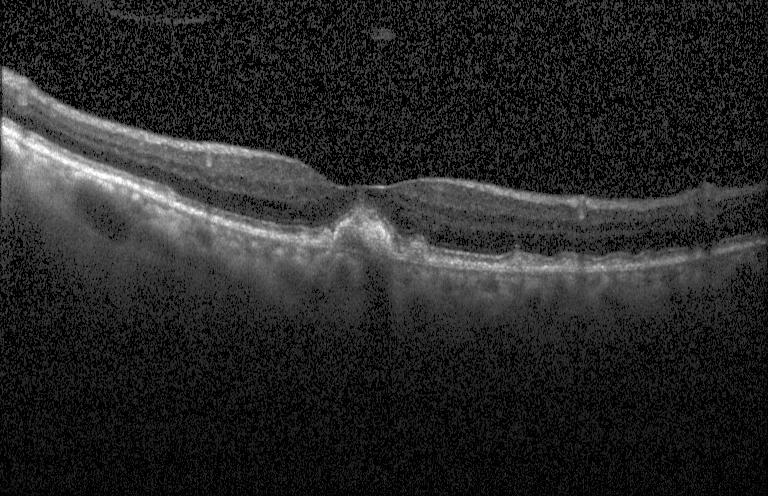 OCT B-scan showing choroidal neovascularization.